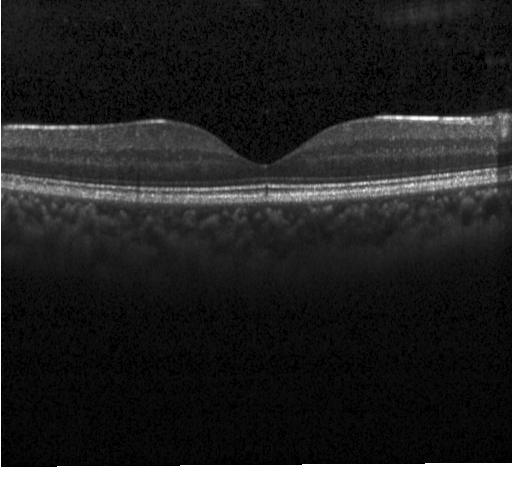

Retinal OCT cross-section; spectral-domain optical coherence tomography
Neither choroidal neovascularization, diabetic macular edema, nor drusen.